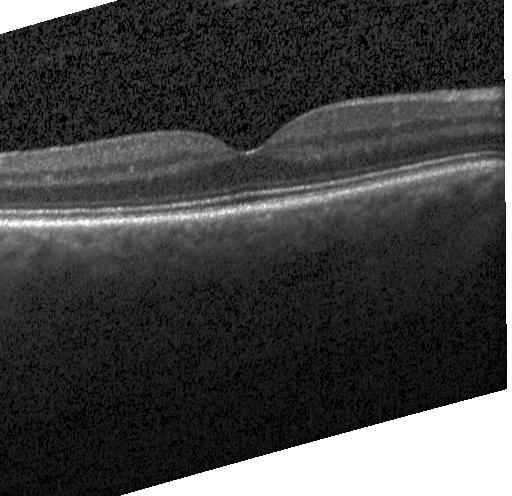

Through the macula; OCT B-scan; Heidelberg Spectralis; SD-OCT
Diagnosis: no choroidal neovascularization, no diabetic macular edema, and no drusen.